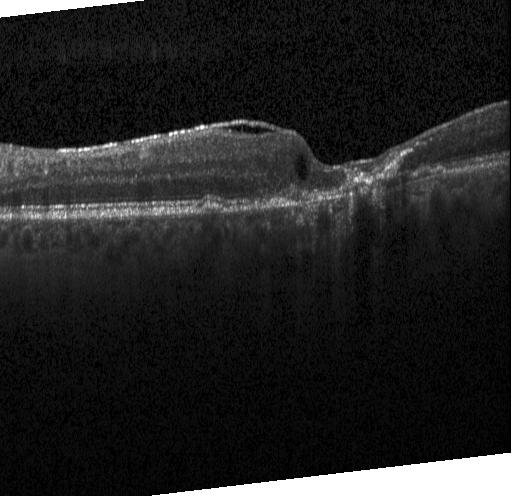

Retinal OCT cross-section
Impression: CNV.